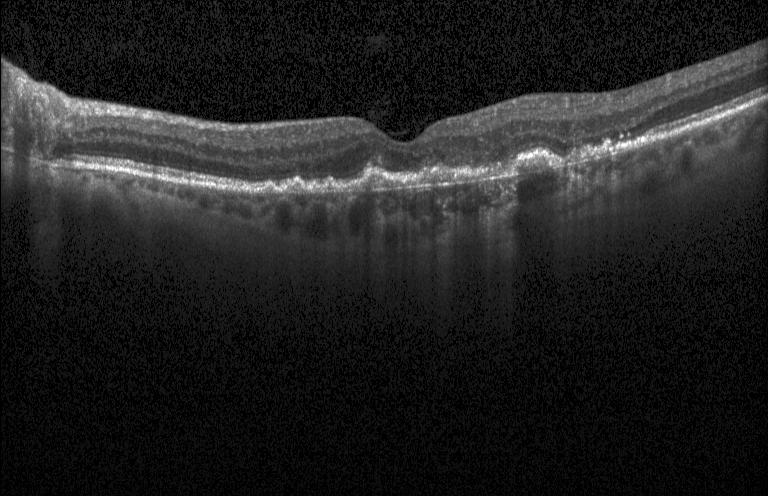 OCT B-scan
Diagnosis: a choroidal neovascular membrane.